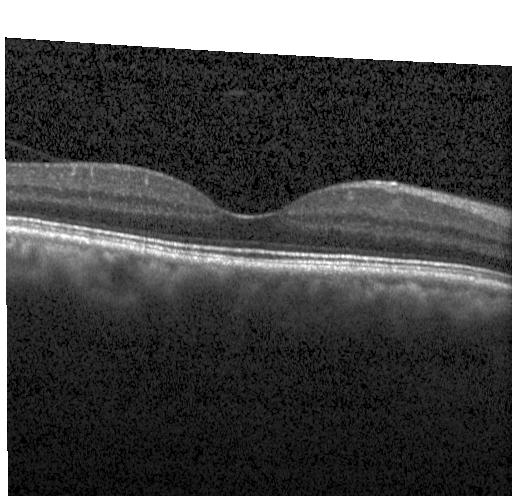
OCT B-scan
Diagnosis: no evidence of choroidal neovascularization, diabetic macular edema, or drusen.